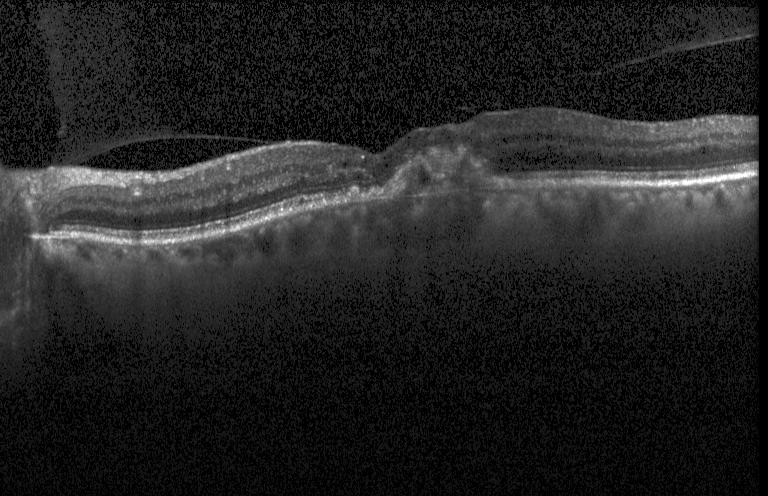 OCT line scan
Assessment: CNV.